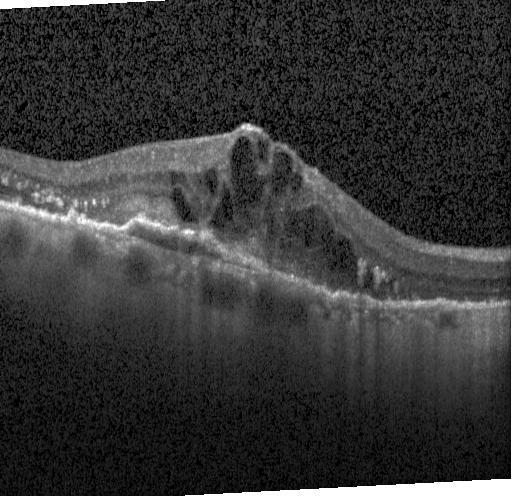 Instrument: Heidelberg Spectralis · spectral-domain OCT · through the macula · OCT line scan. A choroidal neovascular membrane.